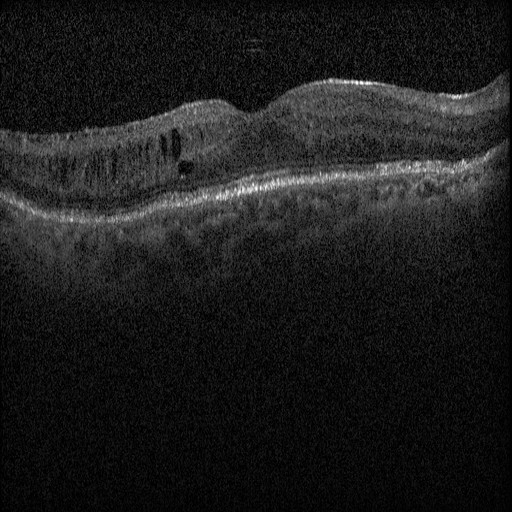 Through the macula, retinal OCT B-scan.
Diabetic macular edema (DME).